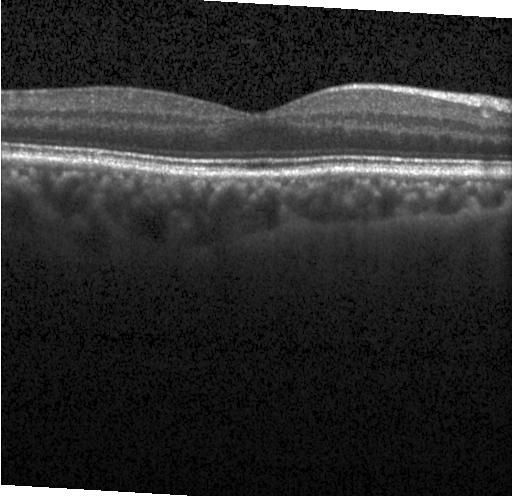 Spectral-domain OCT B-scan: no evidence of choroidal neovascularization, diabetic macular edema, or drusen.